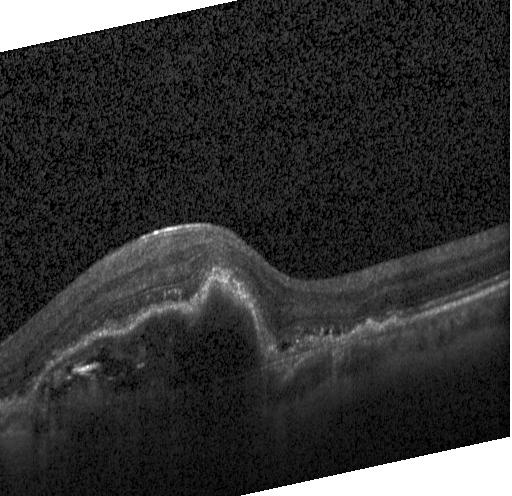

Choroidal neovascularization (CNV).